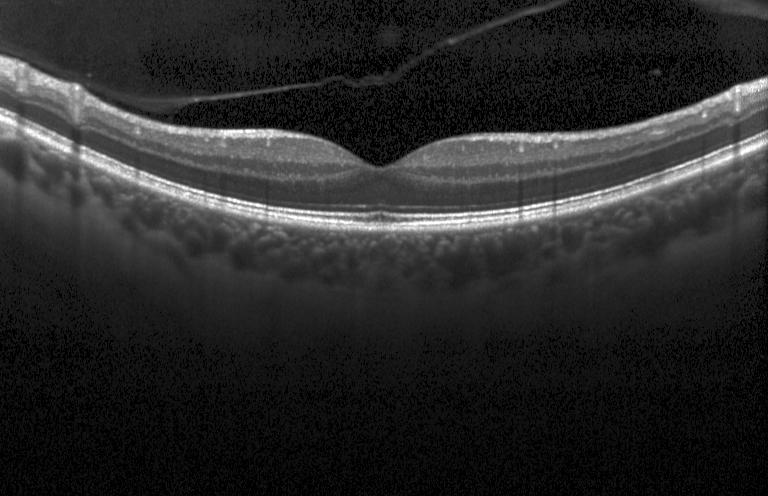

Acquired on a Heidelberg Spectralis · spectral-domain optical coherence tomography · optical coherence tomography scan · macular scan. Impression: neither choroidal neovascularization, diabetic macular edema, nor drusen.